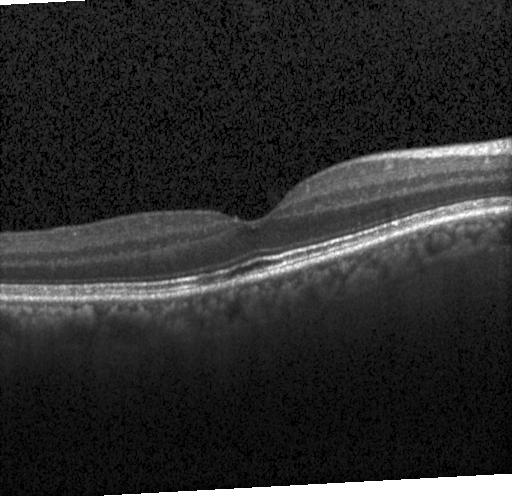
Heidelberg Spectralis. Spectral-domain OCT. OCT B-scan. Macular scan.
Diagnosis: no evidence of choroidal neovascularization, diabetic macular edema, or drusen.